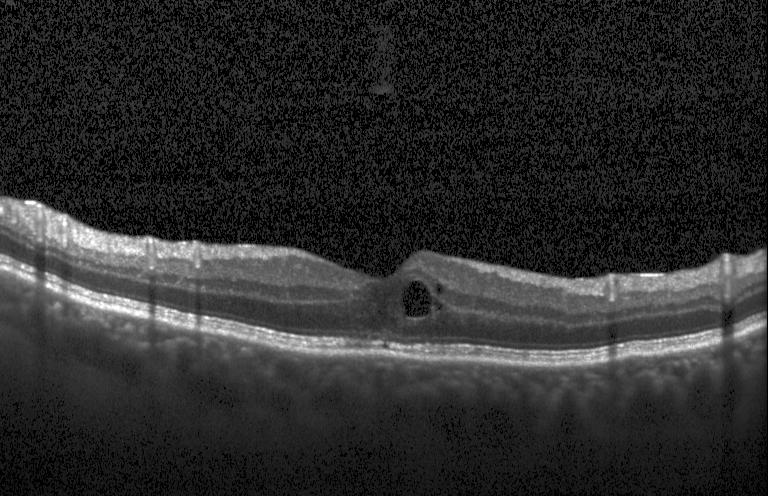

Diabetic macular edema (DME).